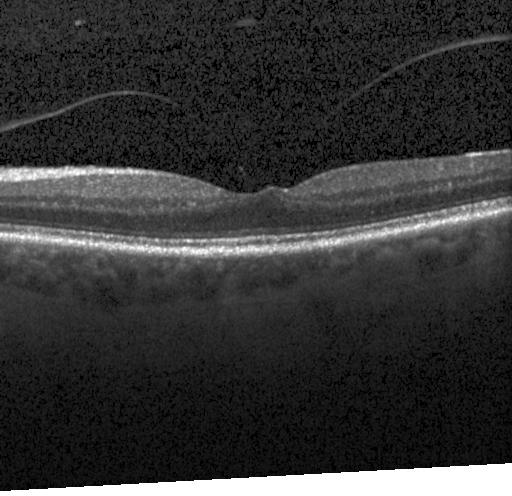 Finding: neither choroidal neovascularization, diabetic macular edema, nor drusen.